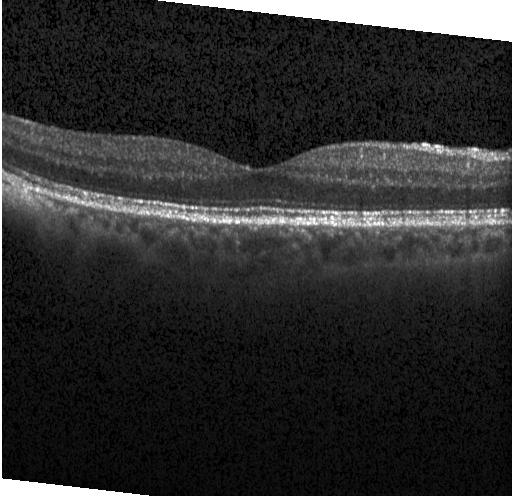
Centered on the fovea. OCT line scan.
Diagnosis: no evidence of choroidal neovascularization, diabetic macular edema, or drusen.